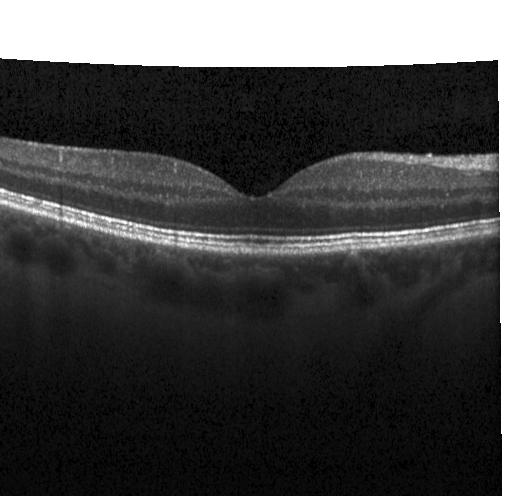
SD-OCT; Heidelberg Spectralis OCT system; retinal OCT cross-section.
Impression: no CNV, no DME, and no drusen.